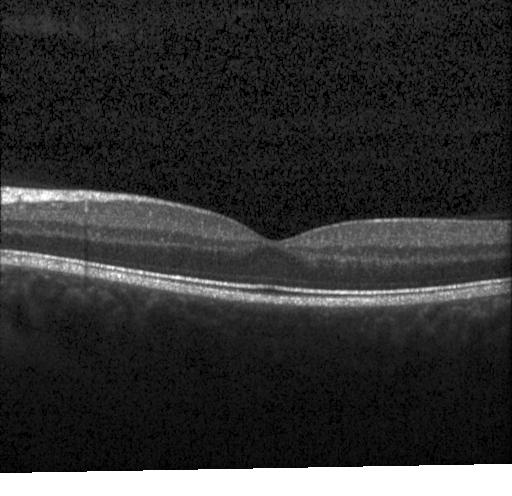
Fovea-centered · instrument: Heidelberg Spectralis · retinal OCT cross-section · spectral-domain OCT — Assessment: no choroidal neovascularization, diabetic macular edema, or drusen.